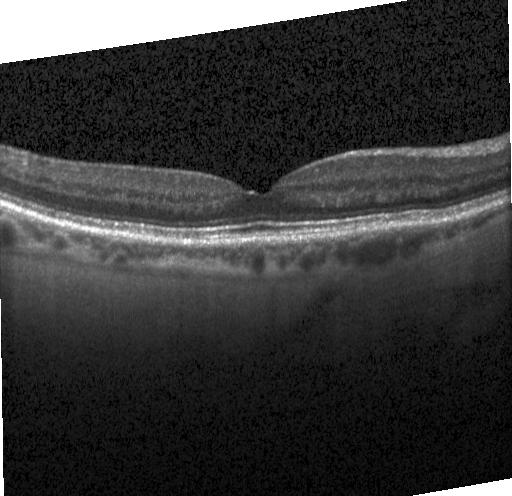
Spectral-domain optical coherence tomography; through the macula; instrument: Heidelberg Spectralis; OCT line scan
Diagnosis: no CNV, DME, or drusen.